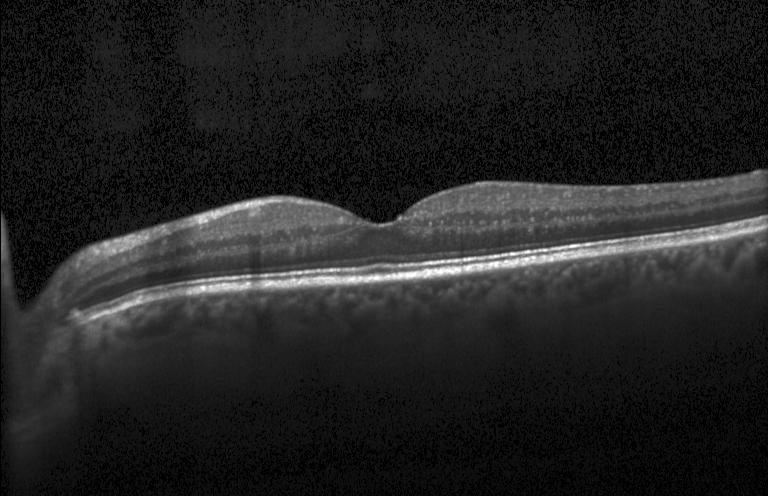
Dx: neither choroidal neovascularization, diabetic macular edema, nor drusen.